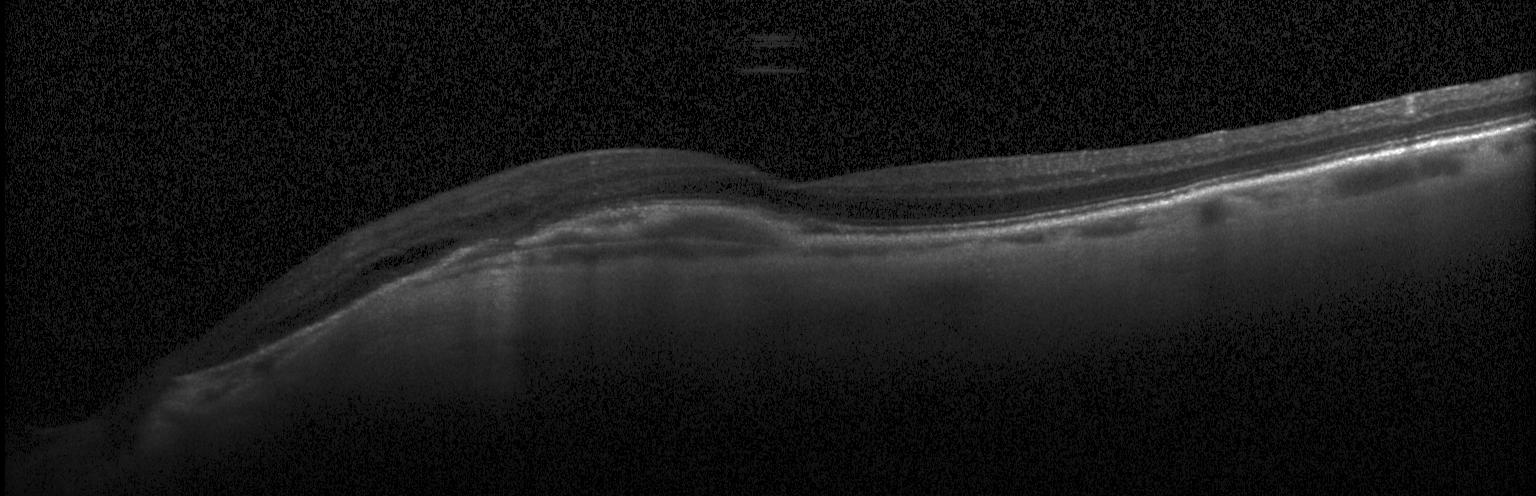
Heidelberg Spectralis. Horizontal scan through the fovea. Spectral-domain optical coherence tomography. Retinal OCT cross-section.
This B-scan demonstrates a choroidal neovascular membrane.